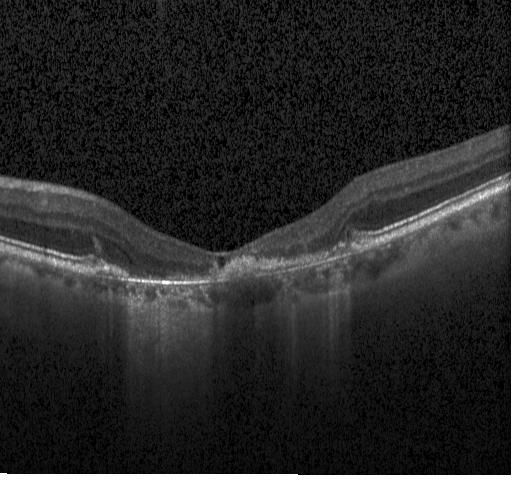

Spectral-domain optical coherence tomography. Fovea-centered. Acquired on a Heidelberg Spectralis. OCT B-scan
Diagnosis: a choroidal neovascular membrane.